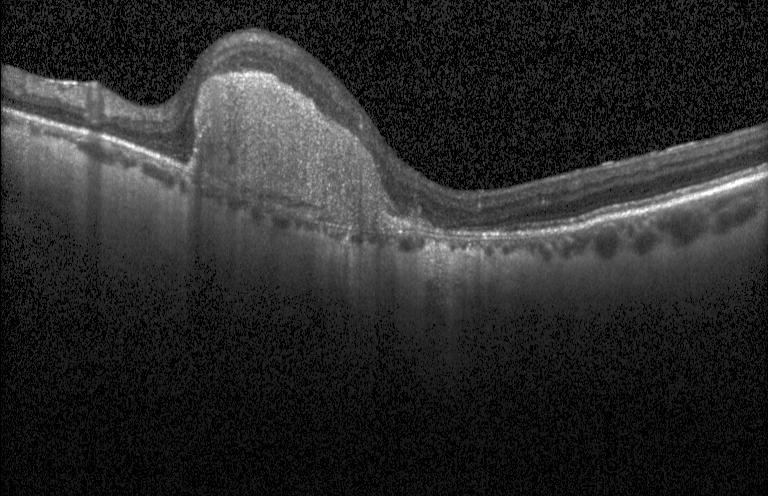 Optical coherence tomography B-scan. Impression: choroidal neovascularization (CNV).